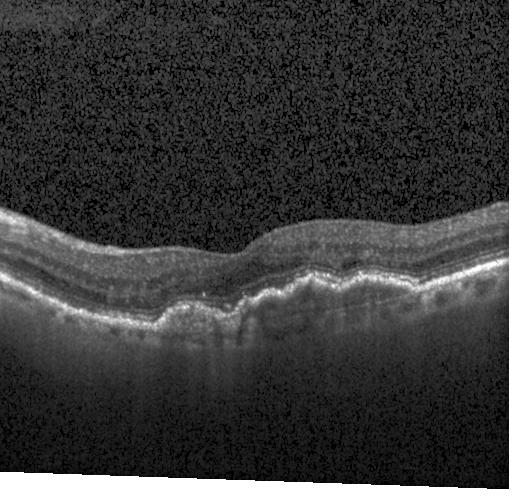

A choroidal neovascular membrane.